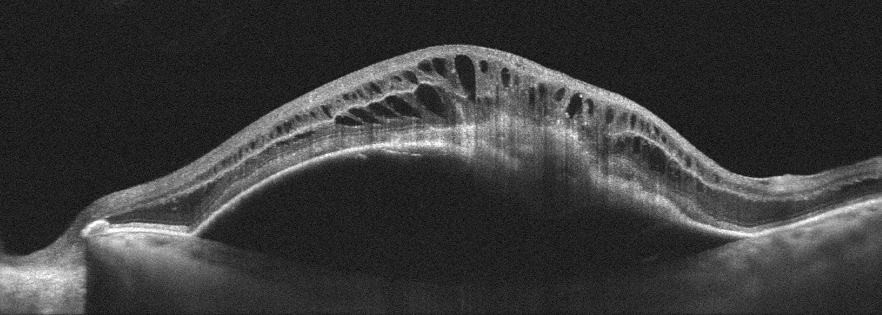

OS; optical coherence tomography scan. Diagnosis: age-related macular degeneration.